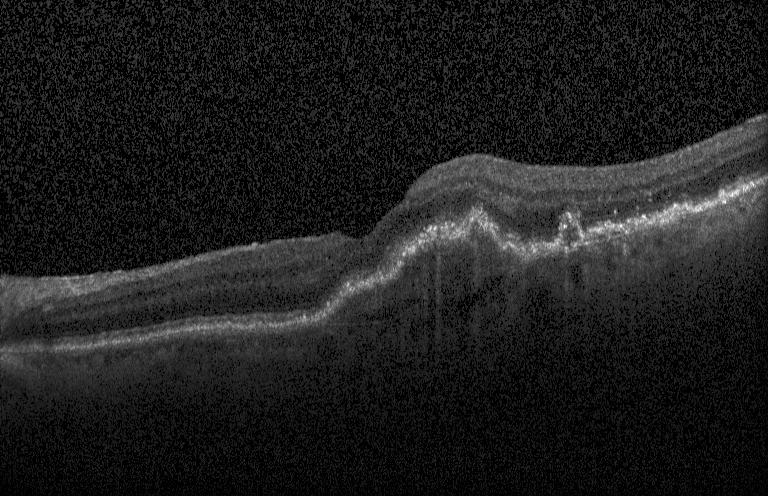
Instrument: Heidelberg Spectralis; centered on the fovea; OCT B-scan; spectral-domain optical coherence tomography
Dx: a choroidal neovascular membrane.